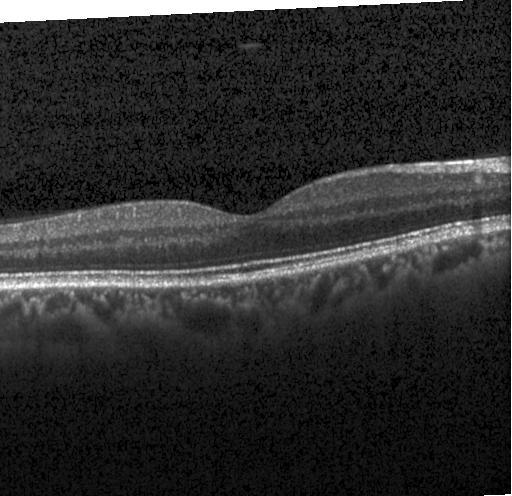
Diagnosis: neither choroidal neovascularization, diabetic macular edema, nor drusen.